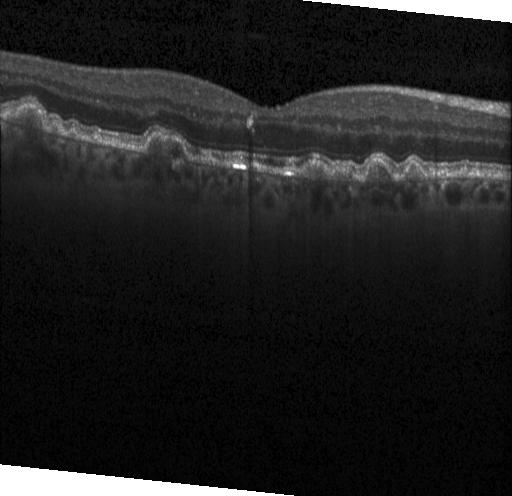

Diagnosis: sub-RPE drusenoid deposits.